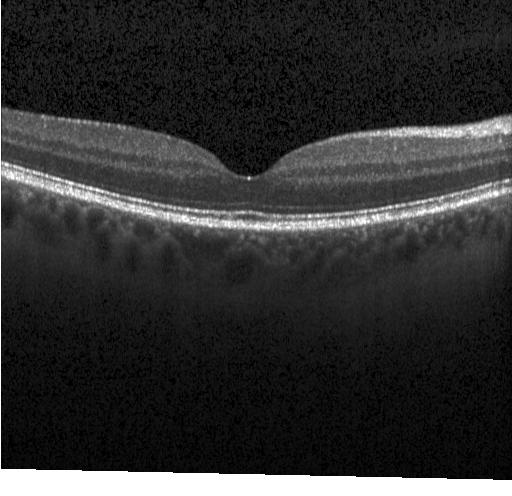

OCT finding: no evidence of choroidal neovascularization, diabetic macular edema, or drusen.